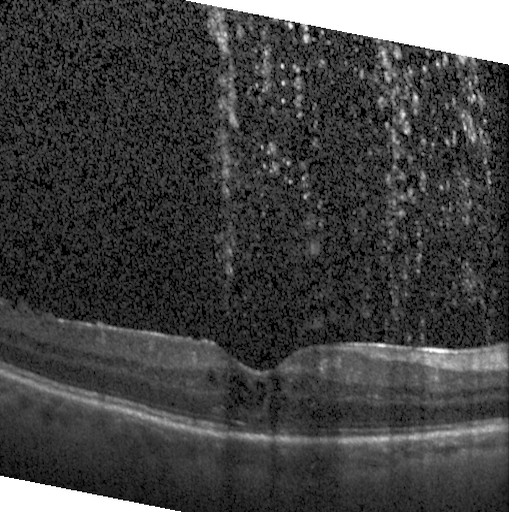

Spectral-domain OCT, optical coherence tomography B-scan — This B-scan demonstrates DME.